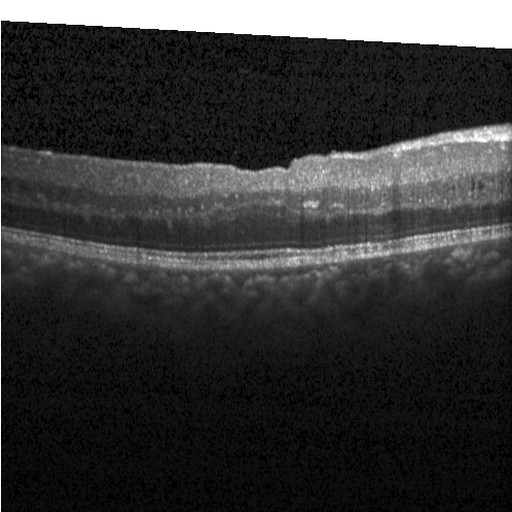

OCT B-scan · horizontal scan through the fovea · instrument: Heidelberg Spectralis
The scan shows diabetic macular edema.